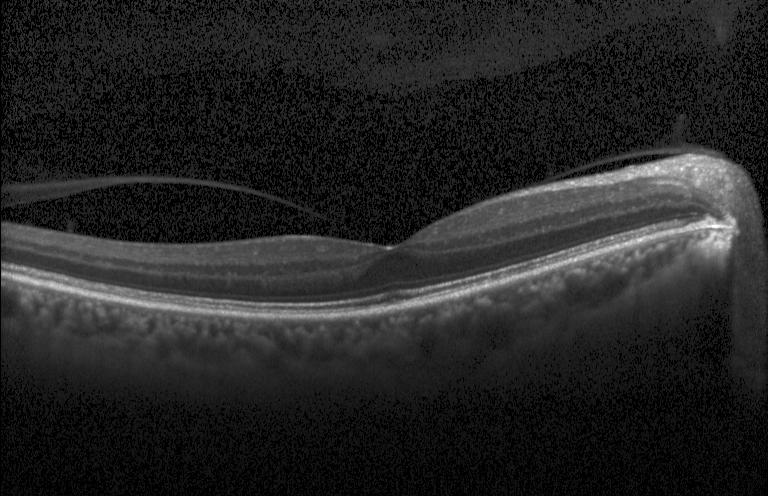

Retinal OCT cross-section showing neither CNV, DME, nor drusen.